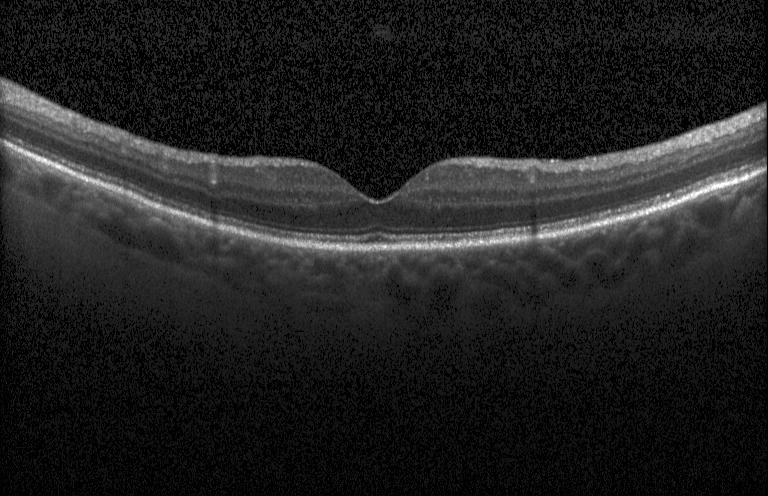 Impression: no CNV, no DME, and no drusen.